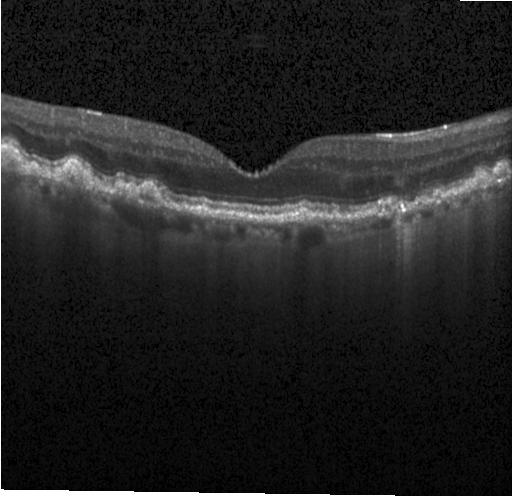 Spectral-domain OCT · fovea-centered · retinal OCT cross-section · acquired on a Heidelberg Spectralis.
Dx: multiple drusen.